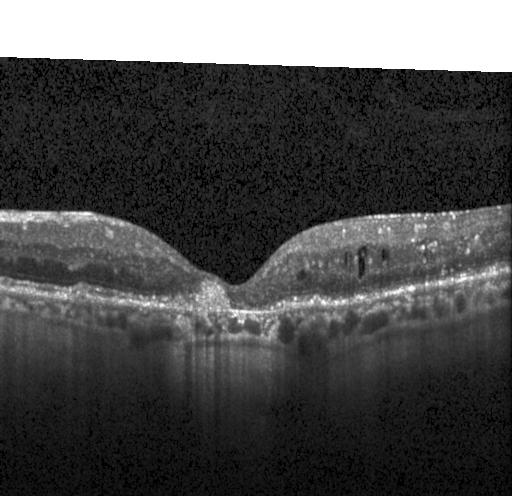 Retinal OCT B-scan · centered on the fovea · Heidelberg Spectralis · spectral-domain optical coherence tomography
Macular OCT: choroidal neovascularization (CNV).